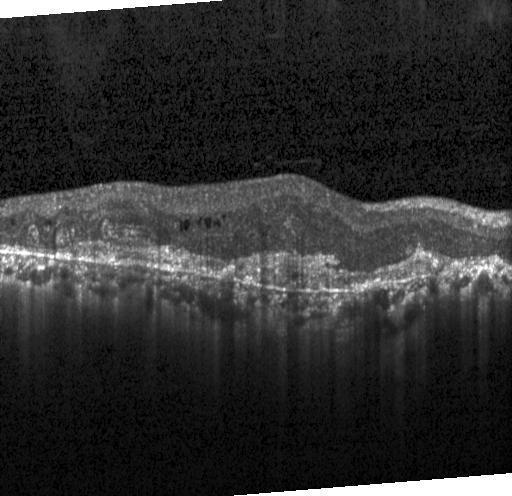
Diagnosis: choroidal neovascularization.